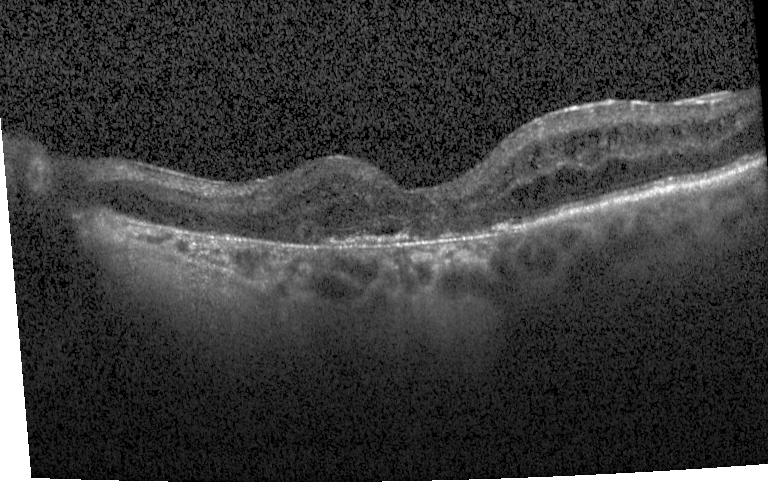
Acquired on a Heidelberg Spectralis. Centered on the fovea. OCT B-scan
Finding: CNV.